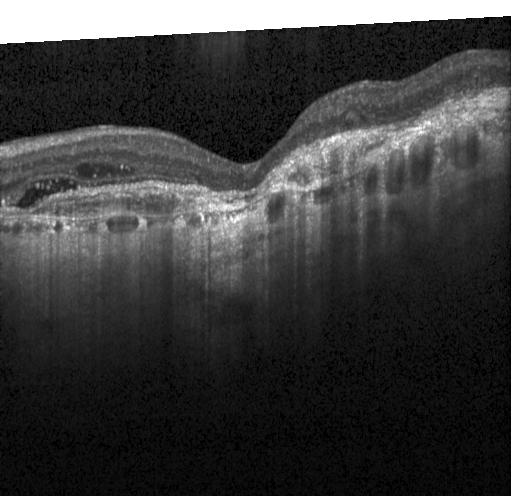
Spectral-domain OCT · horizontal scan through the fovea · Heidelberg Spectralis OCT system · retinal OCT cross-section.
A choroidal neovascular membrane.